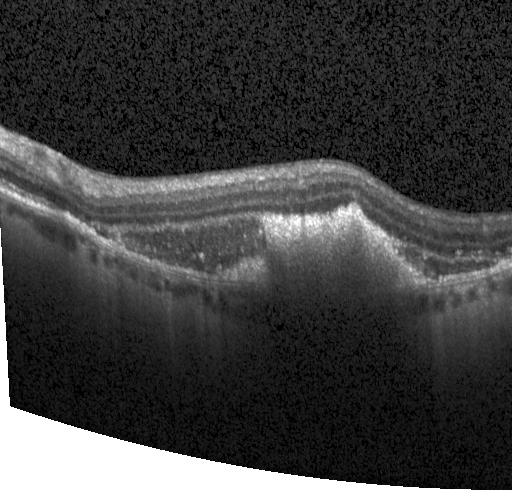 Impression: a choroidal neovascular membrane.